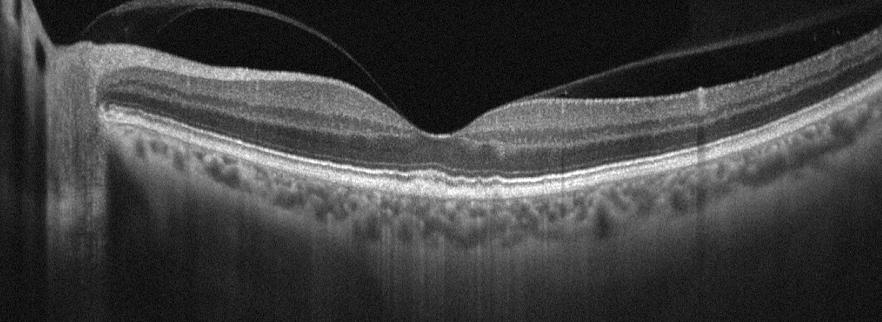
OCT line scan · through the macula · Optovue Avanti RTVue XR.
Impression: AMD.